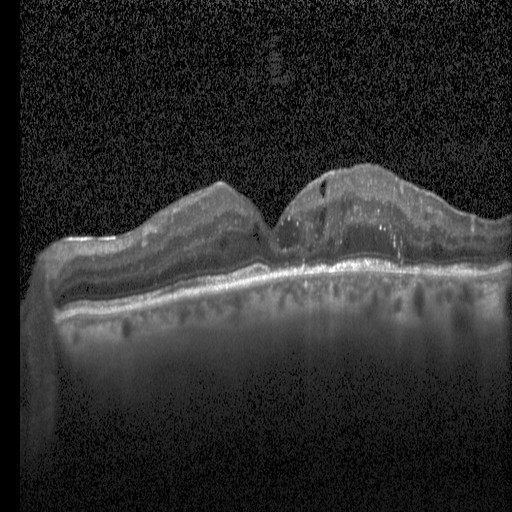

OCT scan showing DME.